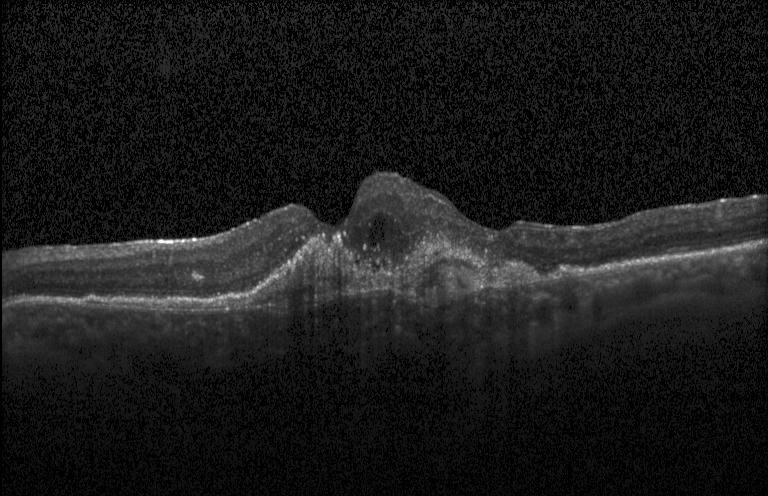
Optical coherence tomography scan — Finding: a choroidal neovascular membrane.